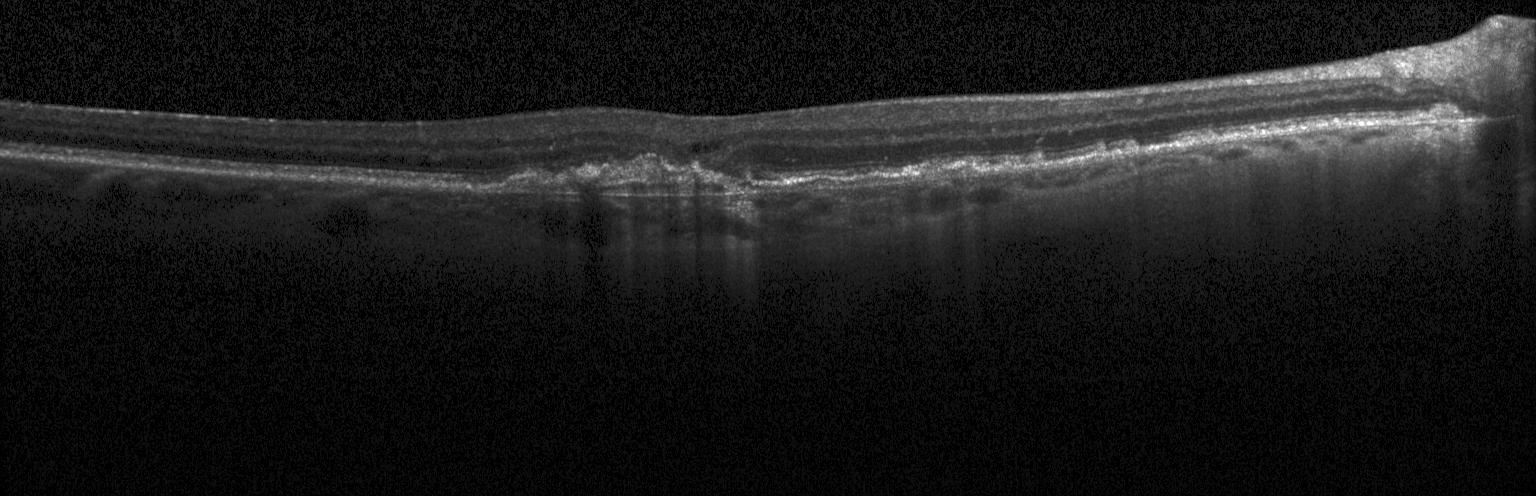

Impression: a choroidal neovascular membrane.